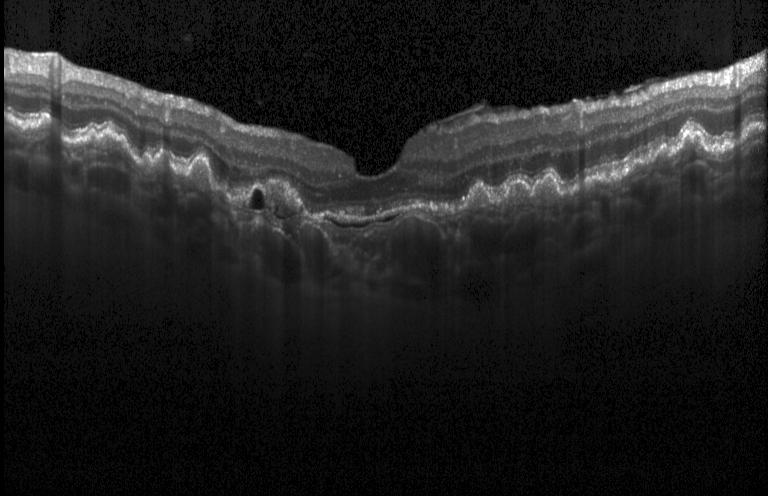 Macular OCT: a choroidal neovascular membrane.